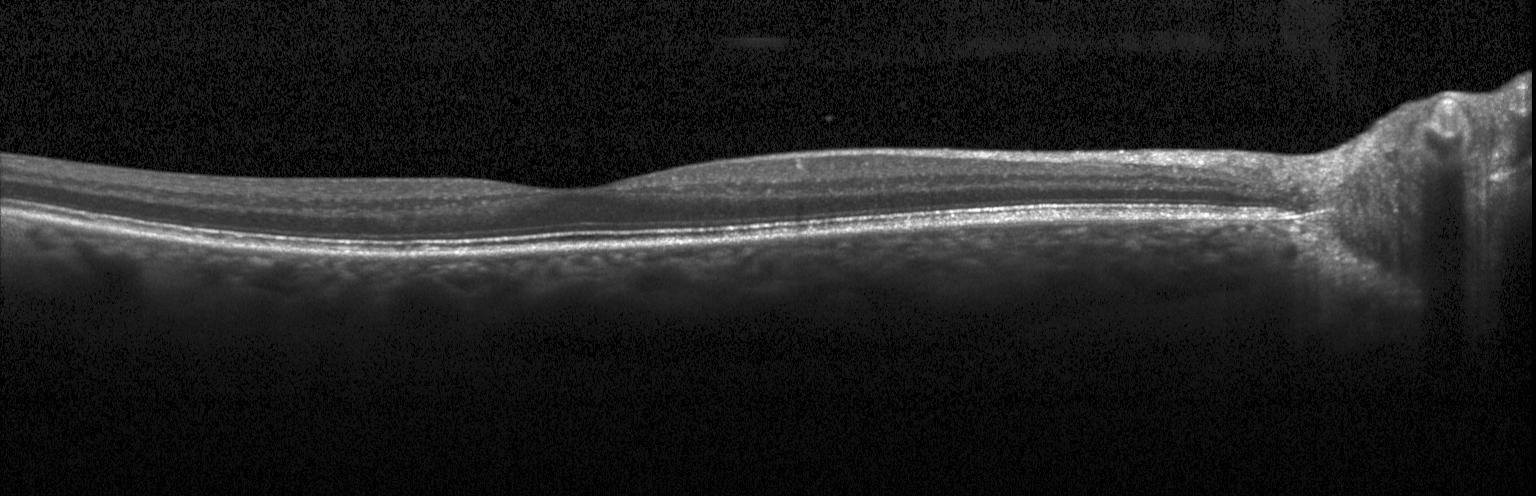 Through the macula, optical coherence tomography scan.
Impression: neither CNV, DME, nor drusen.